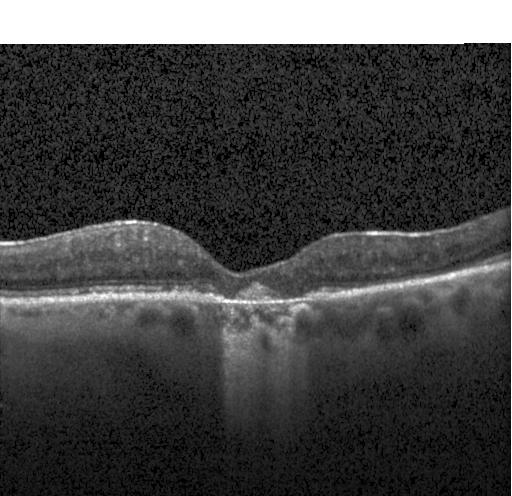

Impression: choroidal neovascularization (CNV).